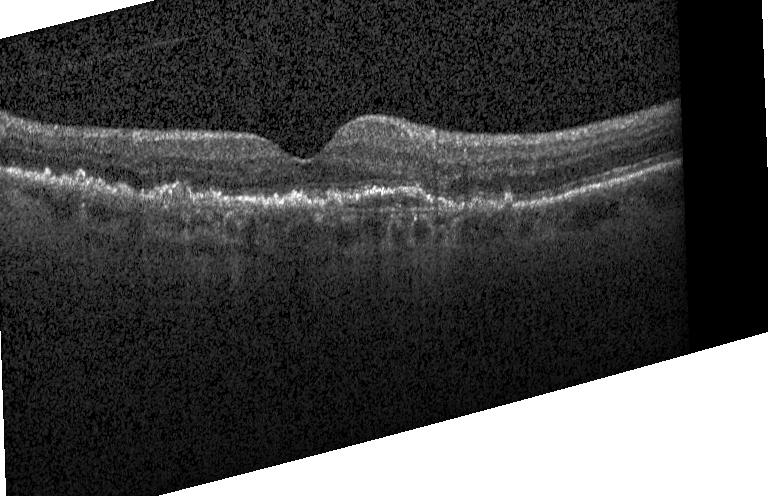 Retinal OCT cross-section, instrument: Heidelberg Spectralis. Choroidal neovascularization.